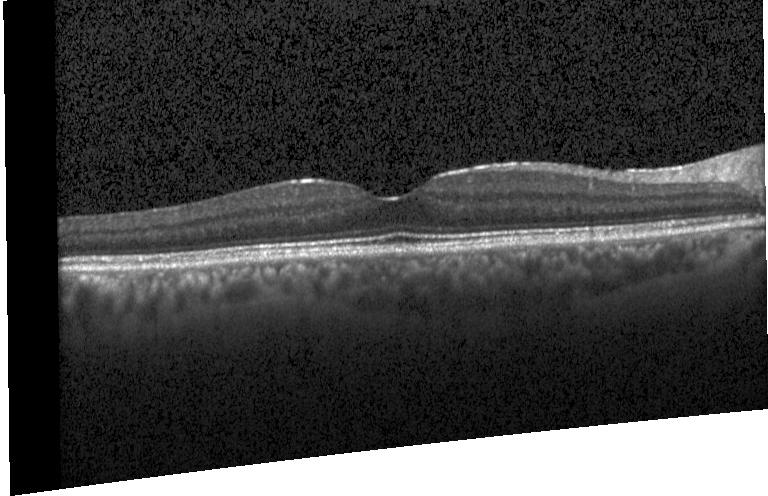

OCT B-scan. The scan shows no choroidal neovascularization, diabetic macular edema, or drusen.